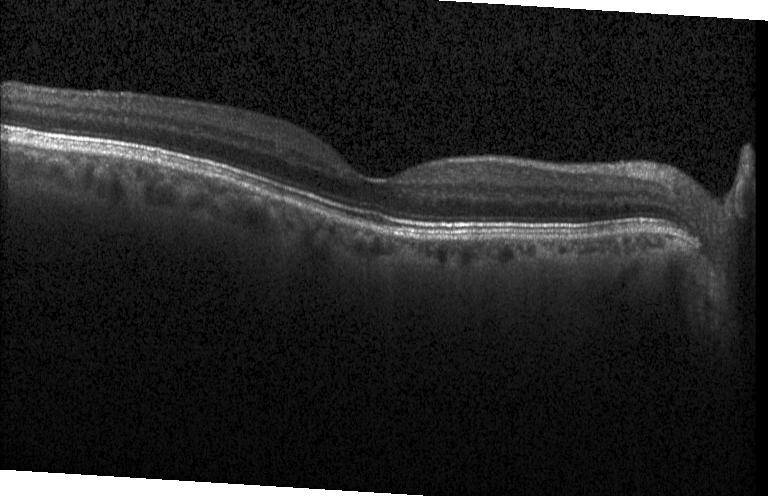

Heidelberg Spectralis, retinal OCT cross-section, SD-OCT.
No CNV, no DME, and no drusen.